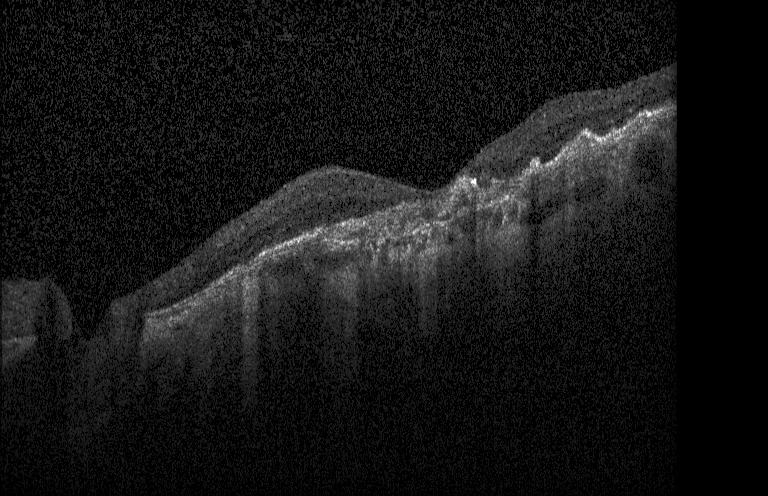
Optical coherence tomography B-scan — Finding: a choroidal neovascular membrane.